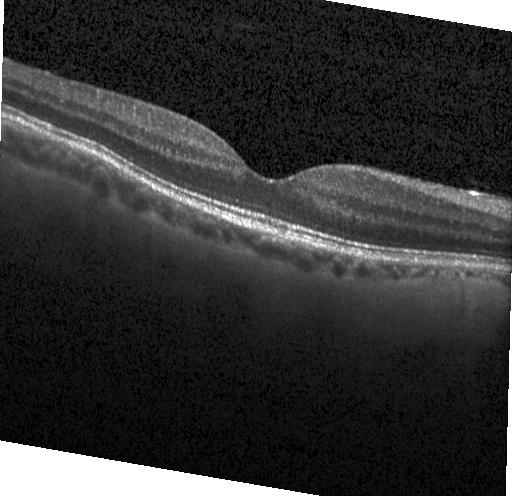 Optical coherence tomography scan; instrument: Heidelberg Spectralis; centered on the fovea — Diagnosis: no evidence of CNV, DME, or drusen.